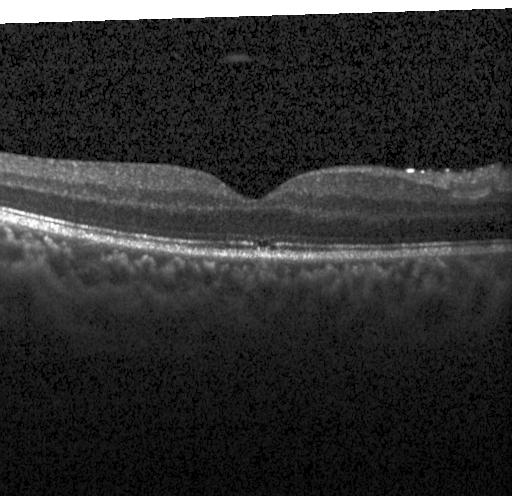

Centered on the fovea. Optical coherence tomography B-scan. Spectral-domain OCT
This B-scan demonstrates no choroidal neovascularization, diabetic macular edema, or drusen.